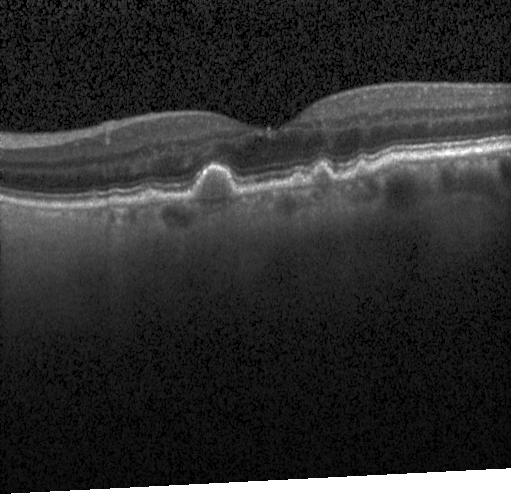 Multiple drusen.